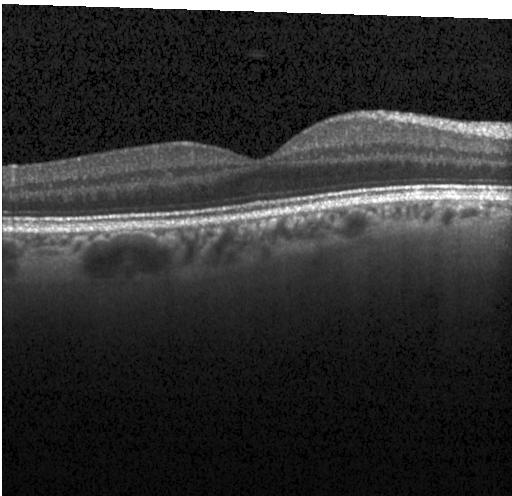 Optical coherence tomography scan. Spectral-domain optical coherence tomography
Diagnosis: no choroidal neovascularization, diabetic macular edema, or drusen.